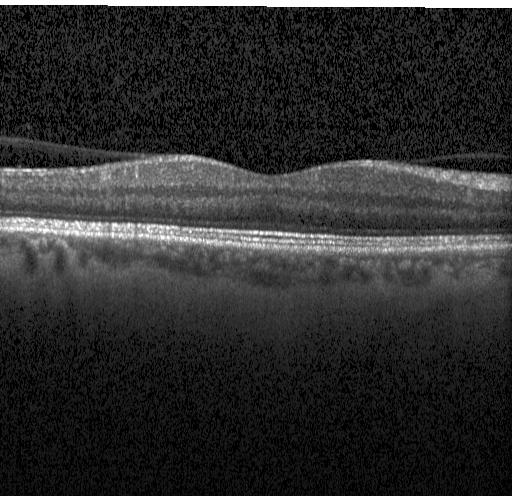 Through the macula, optical coherence tomography B-scan, SD-OCT — Finding: neither choroidal neovascularization, diabetic macular edema, nor drusen.